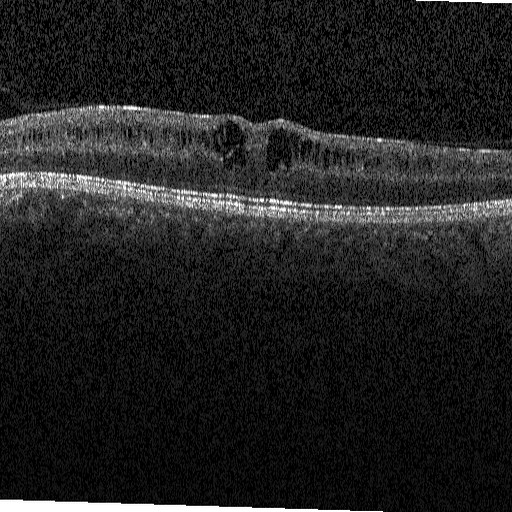

OCT line scan. Finding: diabetic macular edema (DME).